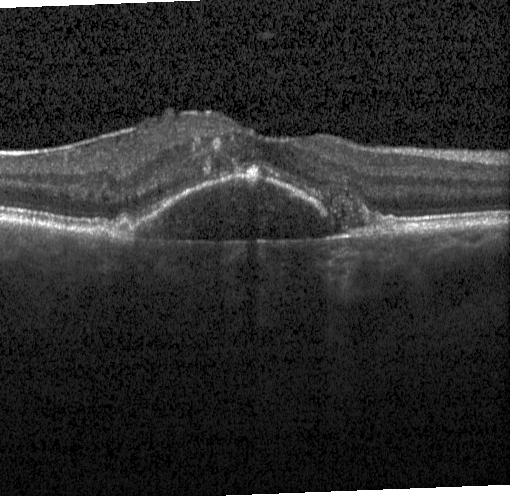

OCT line scan
Diagnosis: a choroidal neovascular membrane.